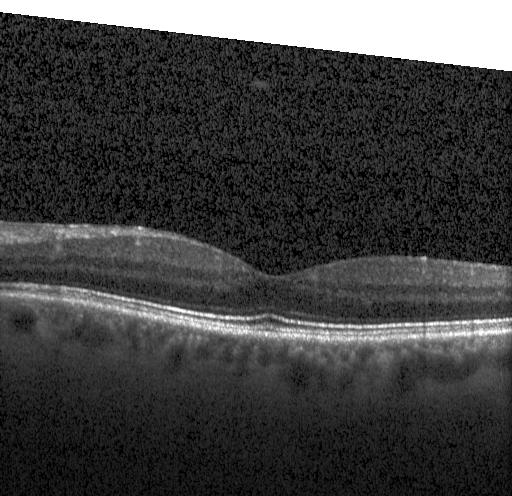 Horizontal scan through the fovea, Heidelberg Spectralis, SD-OCT, retinal OCT cross-section. Assessment: neither CNV, DME, nor drusen.